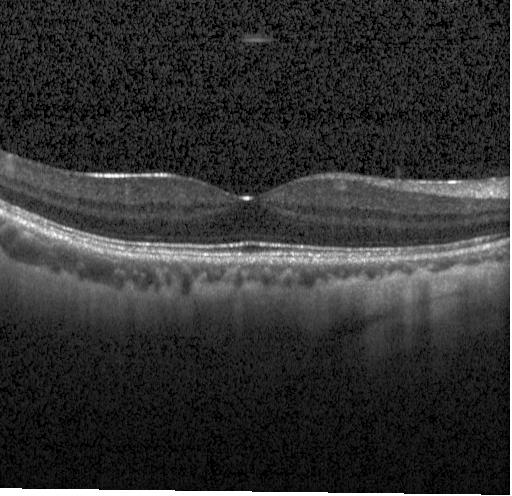
No CNV, no DME, and no drusen.